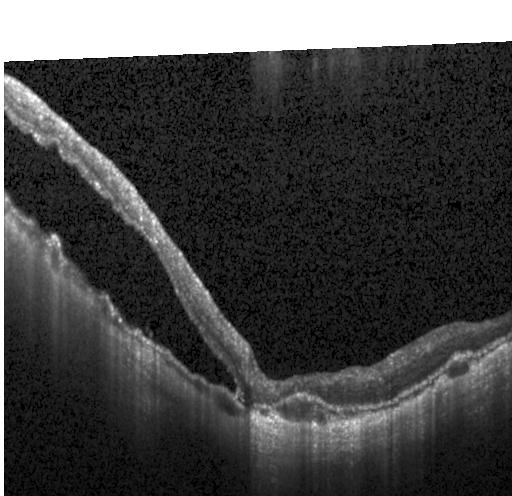
OCT line scan
Impression: a choroidal neovascular membrane.